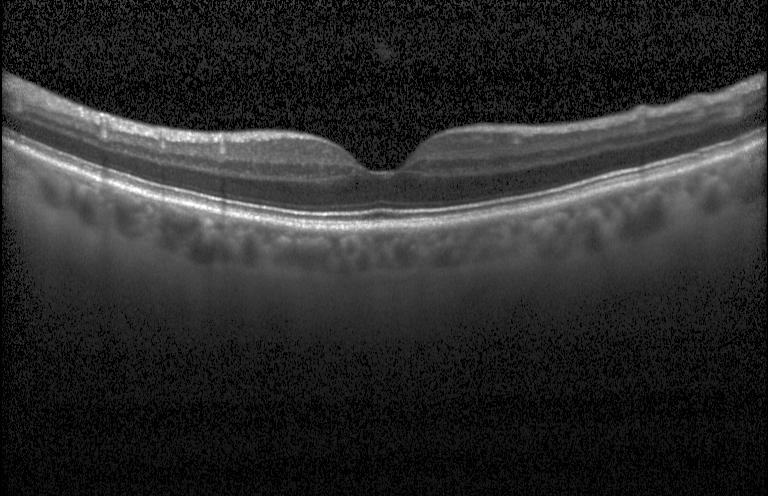

Fovea-centered. SD-OCT. Heidelberg Spectralis OCT system. Optical coherence tomography scan
OCT finding: no choroidal neovascularization, diabetic macular edema, or drusen.